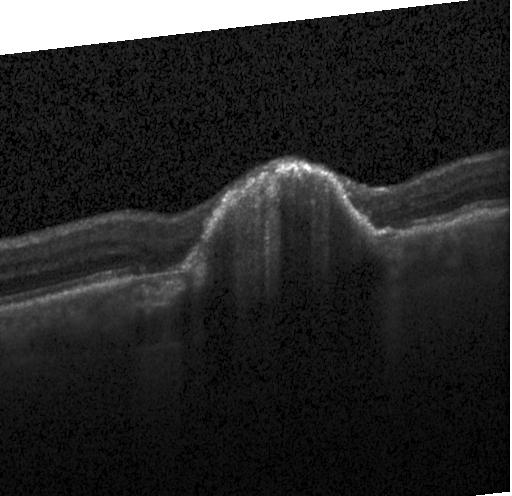 SD-OCT; optical coherence tomography B-scan — Finding: choroidal neovascularization.